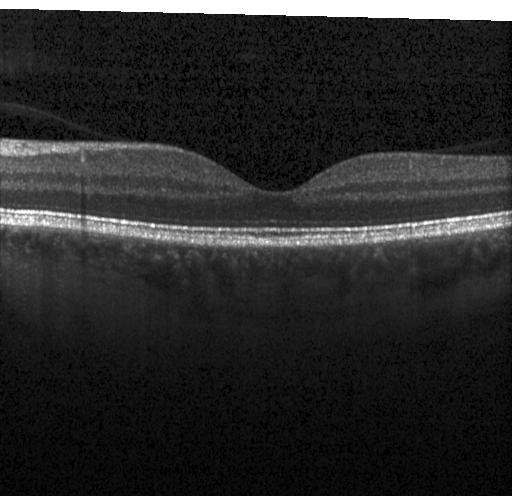
Finding: no choroidal neovascularization, no diabetic macular edema, and no drusen.